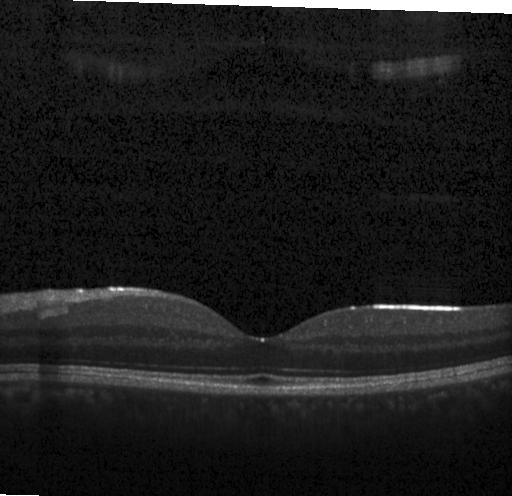
Spectral-domain OCT, retinal OCT B-scan, through the macula
Macular OCT: no CNV, no DME, and no drusen.